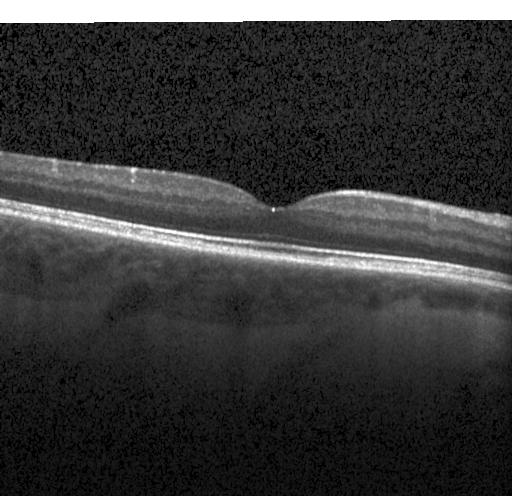 Macular OCT: no evidence of choroidal neovascularization, diabetic macular edema, or drusen.